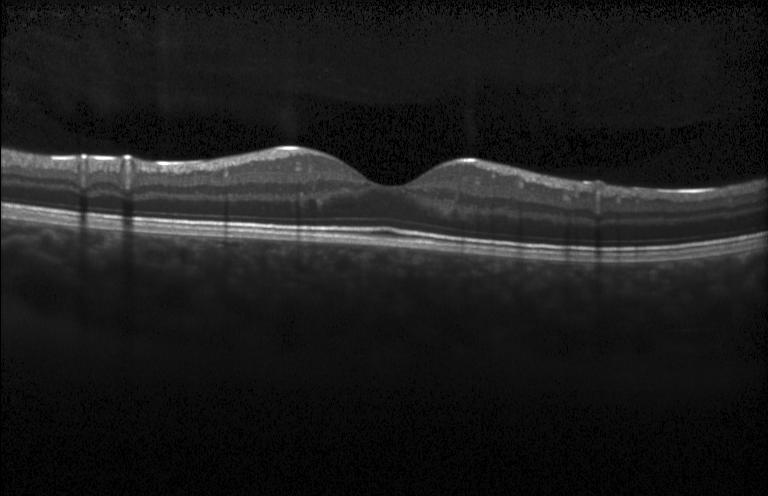

Instrument: Heidelberg Spectralis, spectral-domain optical coherence tomography, retinal OCT B-scan, fovea-centered.
Neither choroidal neovascularization, diabetic macular edema, nor drusen.